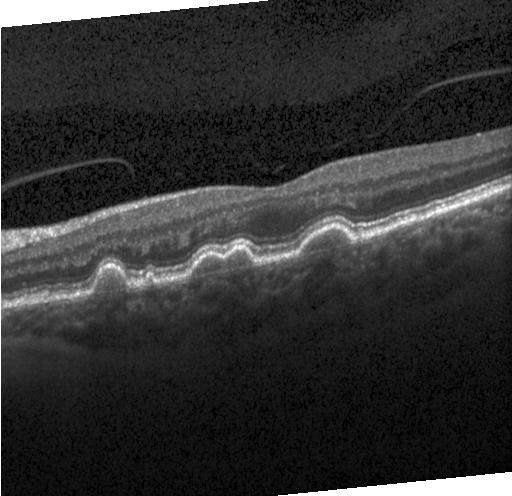 SD-OCT. Heidelberg Spectralis. Optical coherence tomography scan.
This B-scan demonstrates CNV.